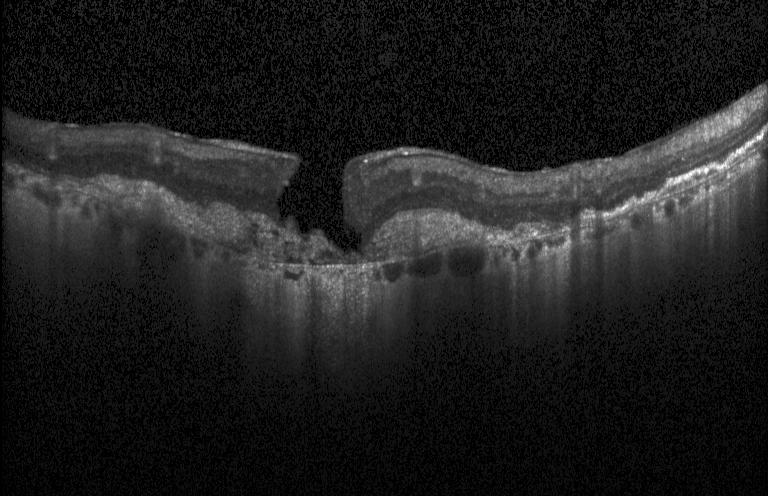
Retinal OCT B-scan. Centered on the fovea. Acquired on a Heidelberg Spectralis. Finding: a choroidal neovascular membrane.